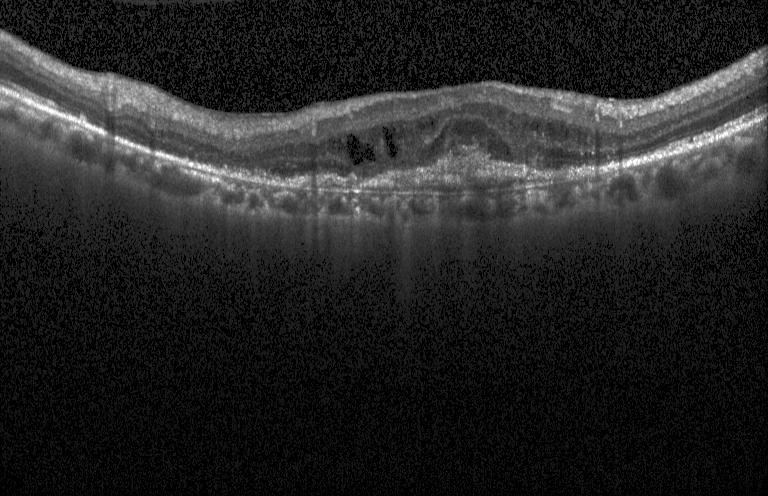 OCT line scan. Impression: choroidal neovascularization.